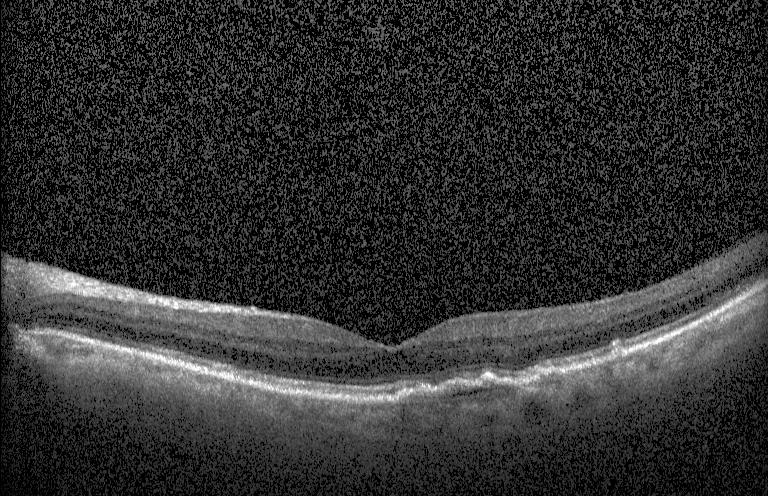 Retinal OCT cross-section.
Assessment: choroidal neovascularization.